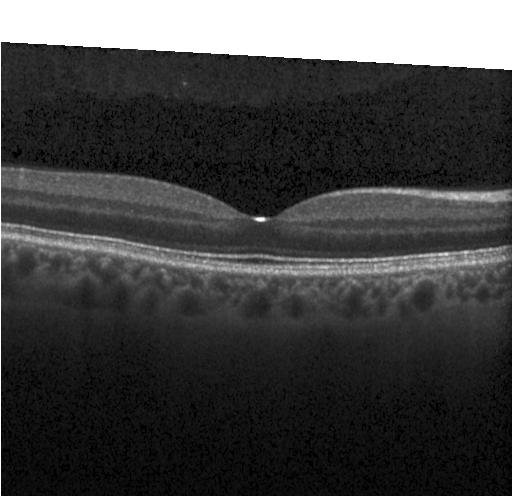 Retinal OCT B-scan. Assessment: no choroidal neovascularization, diabetic macular edema, or drusen.